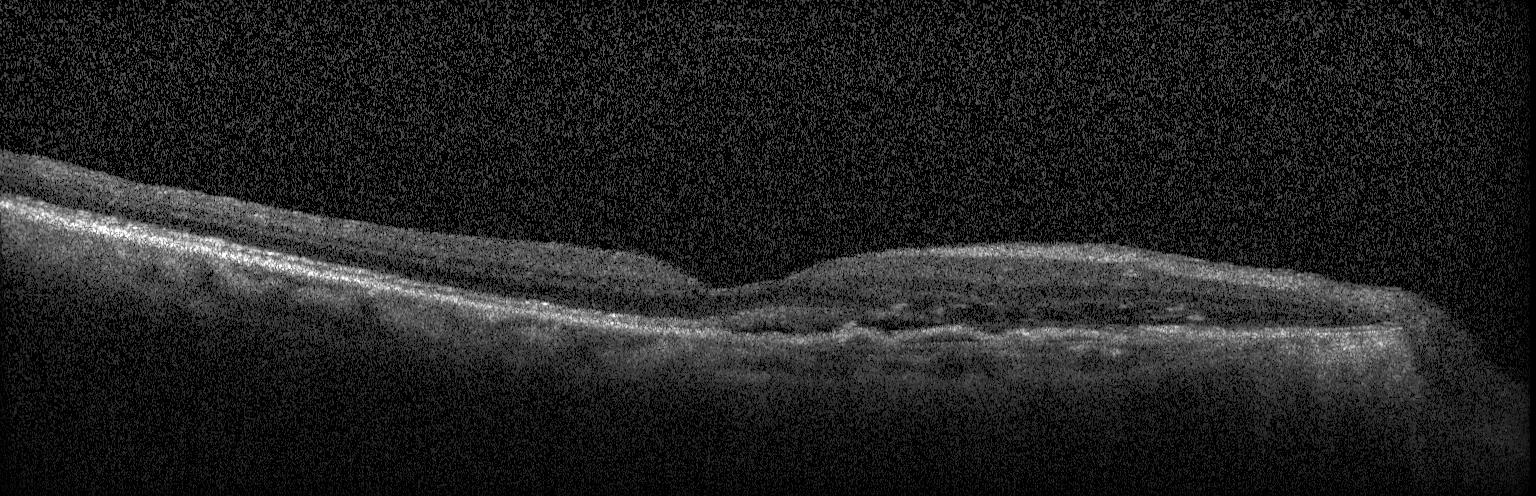
Centered on the fovea · OCT B-scan.
Diagnosis: a choroidal neovascular membrane.